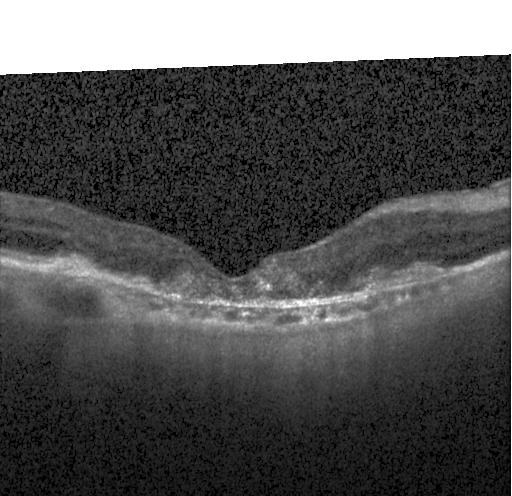

Macular OCT: choroidal neovascularization (CNV).